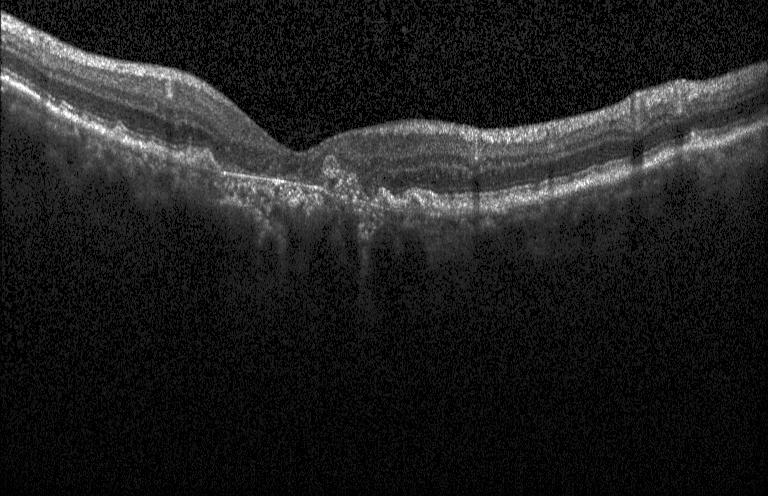 Retinal OCT cross-section — The scan shows choroidal neovascularization.